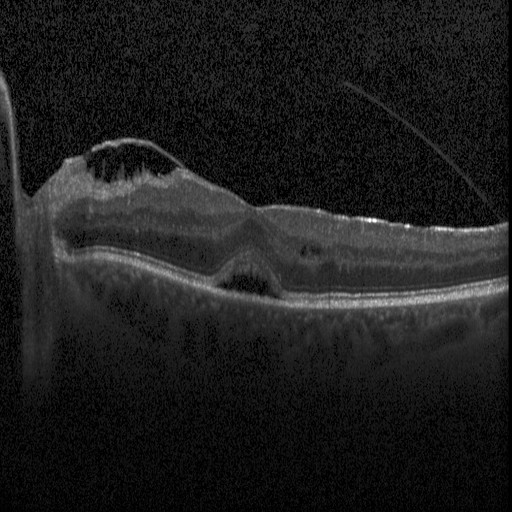 Macular OCT demonstrating DME.